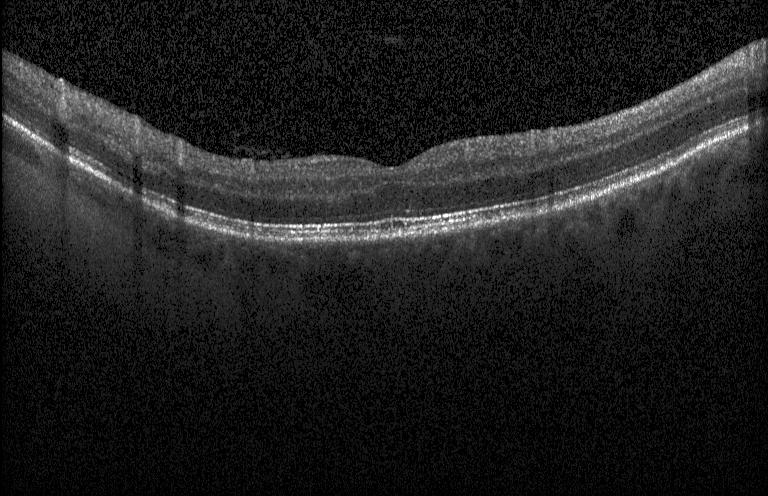 Macular scan. Optical coherence tomography scan. Spectral-domain OCT
No choroidal neovascularization, diabetic macular edema, or drusen.